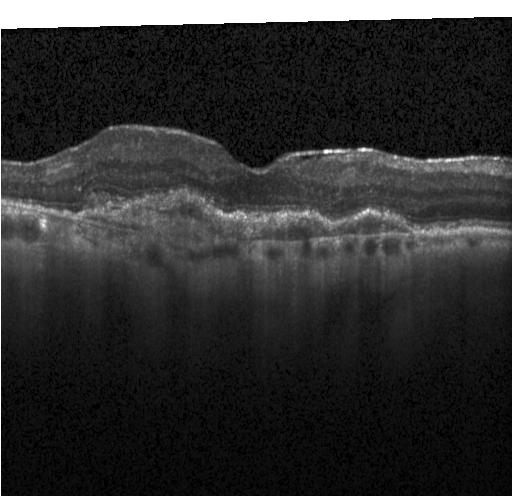

OCT finding: choroidal neovascularization.